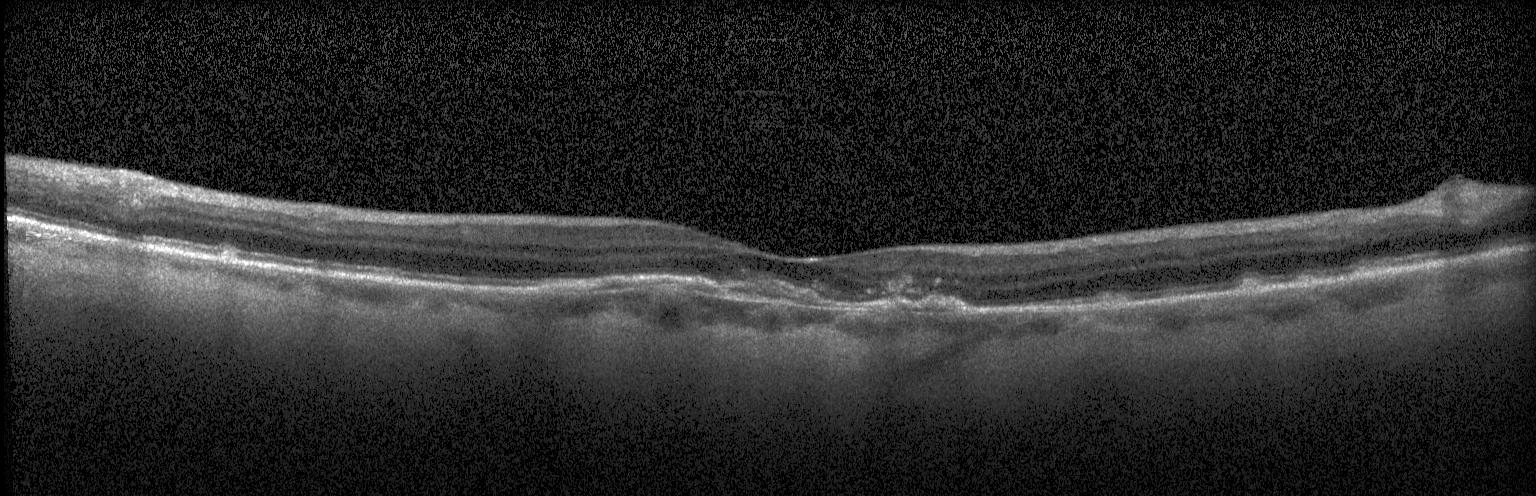 Diagnosis: a choroidal neovascular membrane.